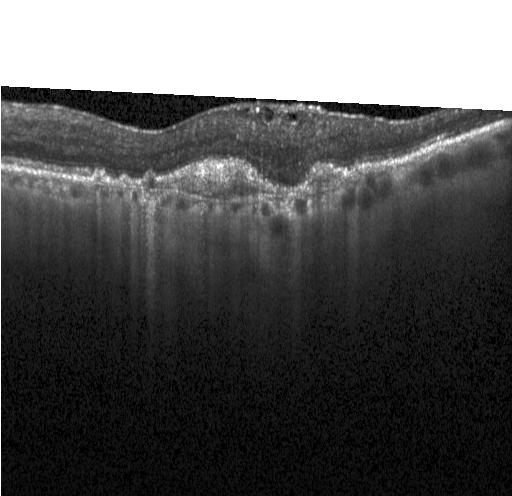

Horizontal scan through the fovea, optical coherence tomography B-scan
This B-scan demonstrates choroidal neovascularization.